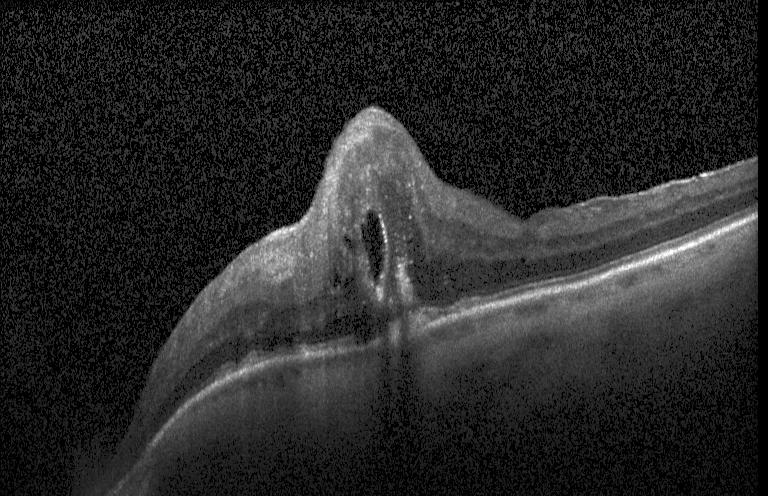

Spectral-domain optical coherence tomography · OCT B-scan · fovea-centered — Assessment: a choroidal neovascular membrane.